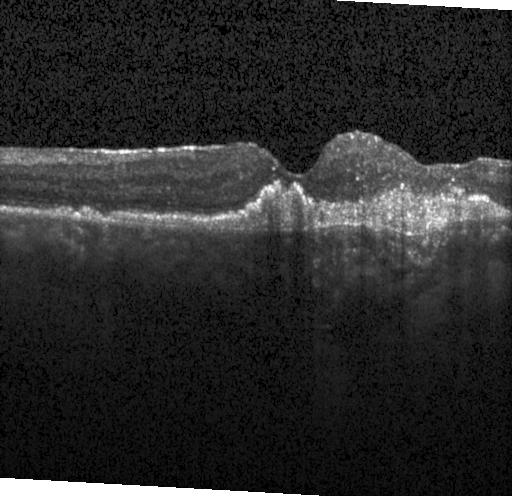 Optical coherence tomography B-scan.
Impression: choroidal neovascularization (CNV).